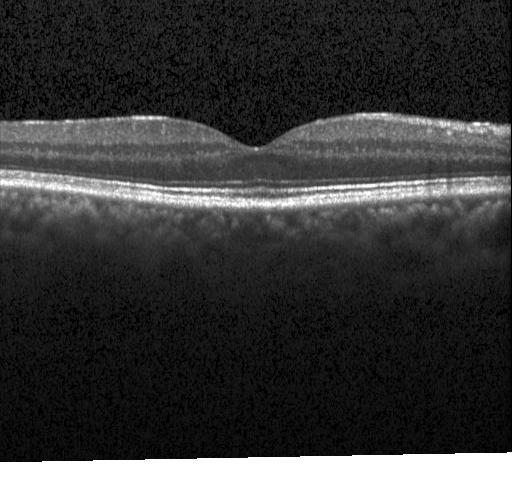 Optical coherence tomography B-scan — Macular OCT: no evidence of CNV, DME, or drusen.